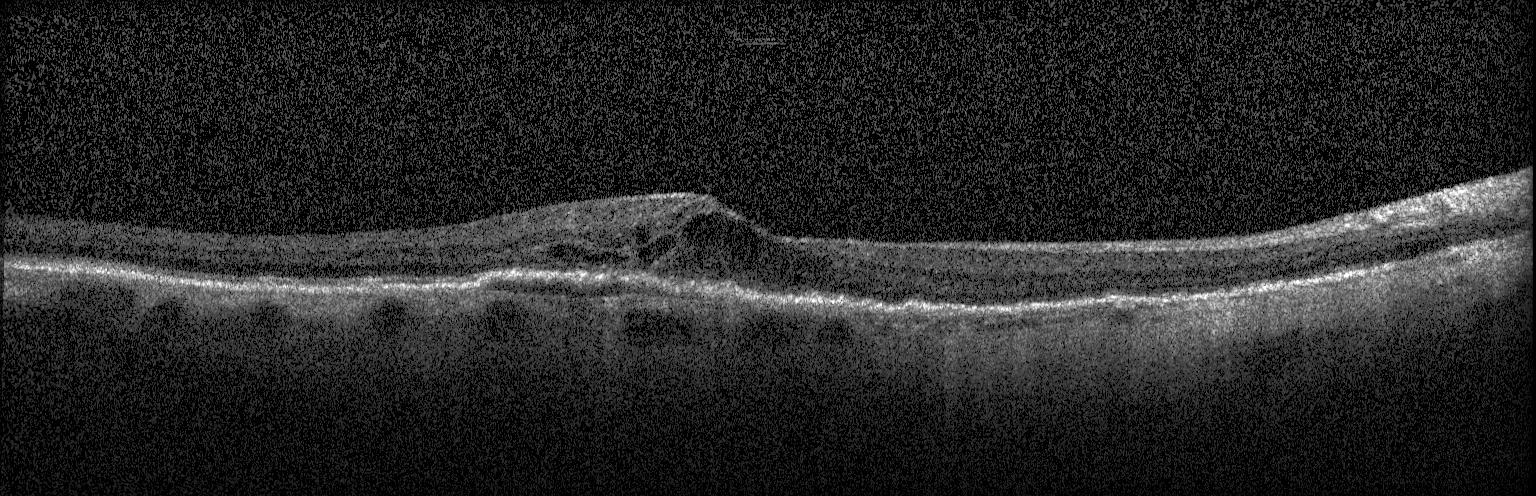 Retinal OCT cross-section — Diagnosis: a choroidal neovascular membrane.